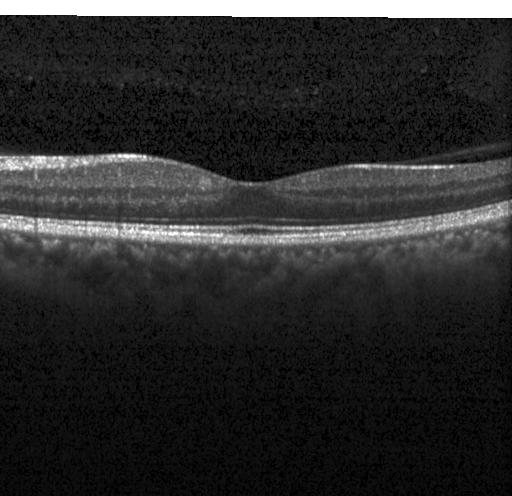

OCT line scan — Diagnosis: no choroidal neovascularization, no diabetic macular edema, and no drusen.